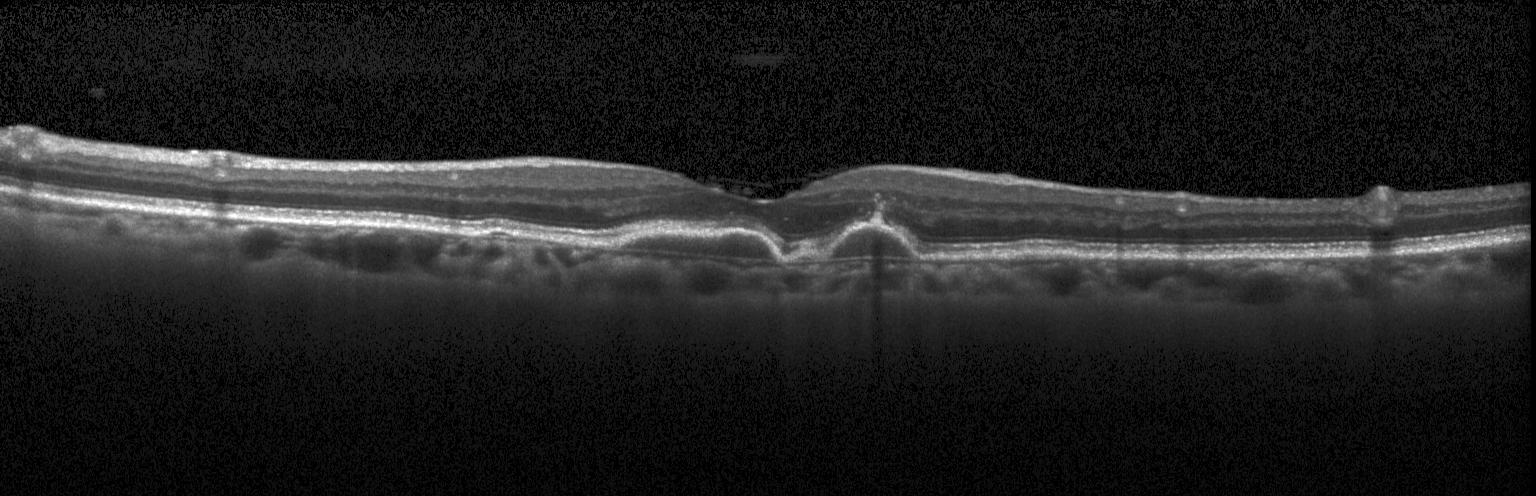
Spectral-domain optical coherence tomography. Centered on the fovea. Optical coherence tomography B-scan
Macular OCT: a choroidal neovascular membrane.